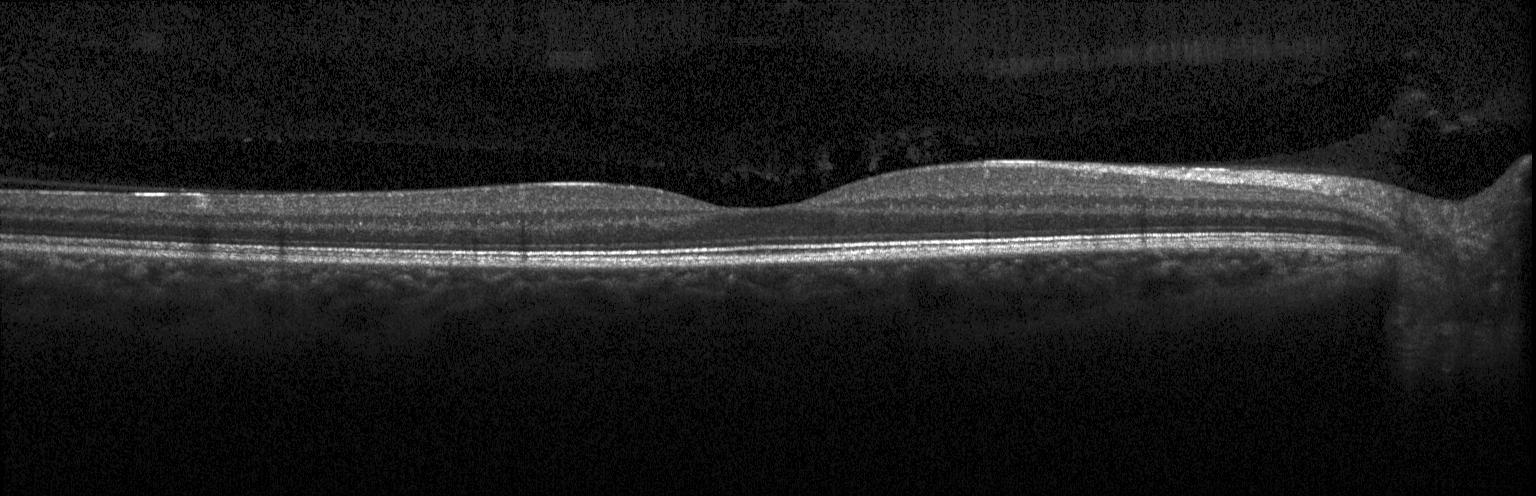 Macular OCT: neither CNV, DME, nor drusen.